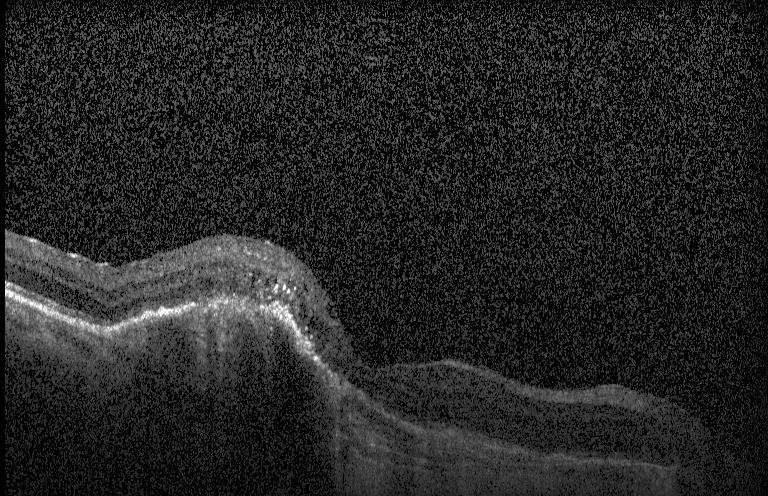

Spectral-domain optical coherence tomography, fovea-centered, retinal OCT B-scan — OCT finding: CNV.